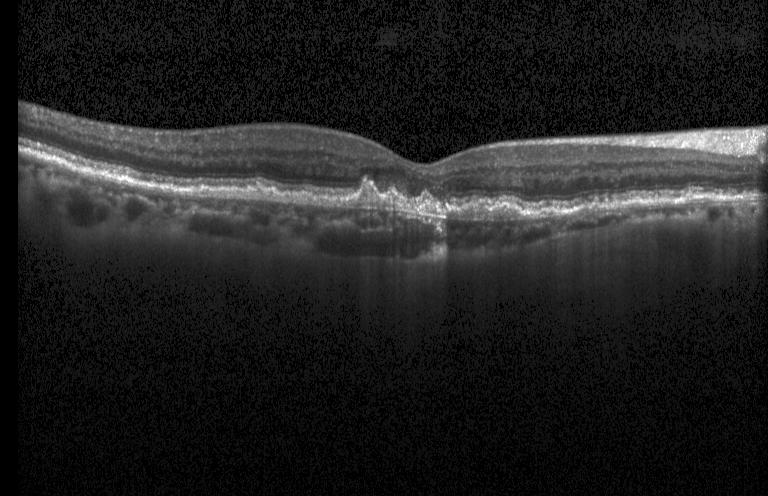 Spectral-domain optical coherence tomography. Heidelberg Spectralis. Fovea-centered. OCT line scan — Finding: a choroidal neovascular membrane.